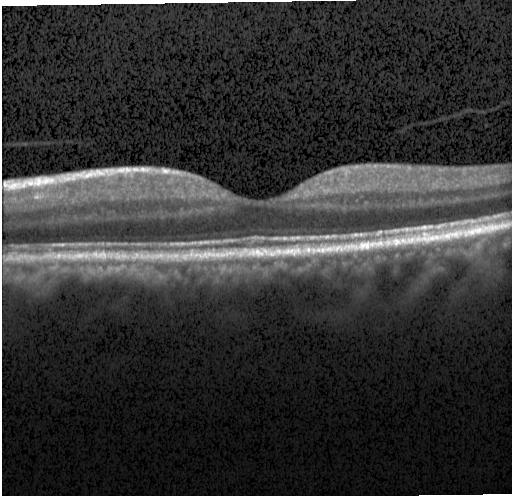 Assessment: no choroidal neovascularization, no diabetic macular edema, and no drusen.